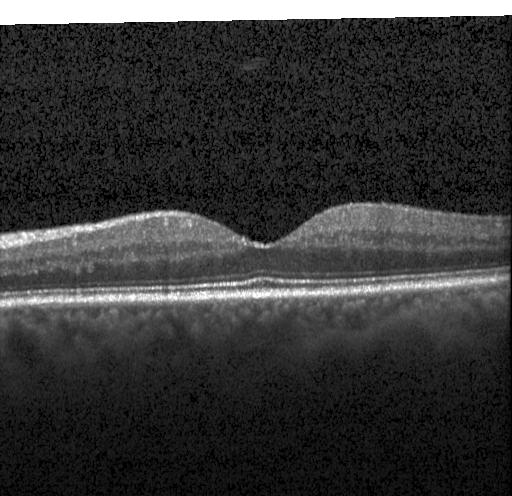 Macular scan. Spectral-domain OCT. Optical coherence tomography scan. Instrument: Heidelberg Spectralis — No choroidal neovascularization, diabetic macular edema, or drusen.